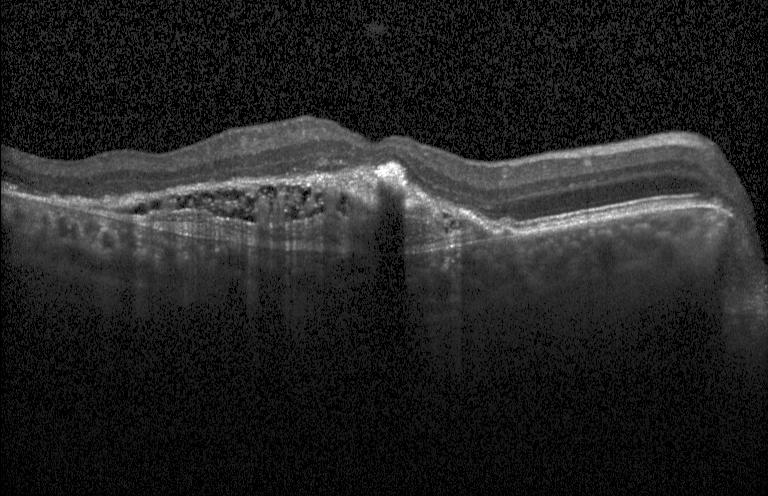

Optical coherence tomography B-scan.
This B-scan demonstrates a choroidal neovascular membrane.